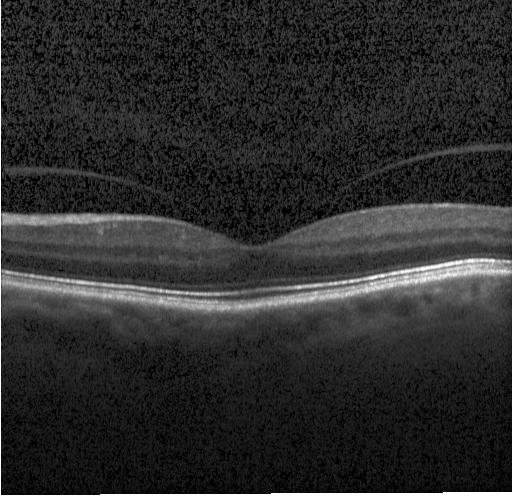

Optical coherence tomography scan; spectral-domain OCT; centered on the fovea; Heidelberg Spectralis
This B-scan demonstrates no choroidal neovascularization, diabetic macular edema, or drusen.